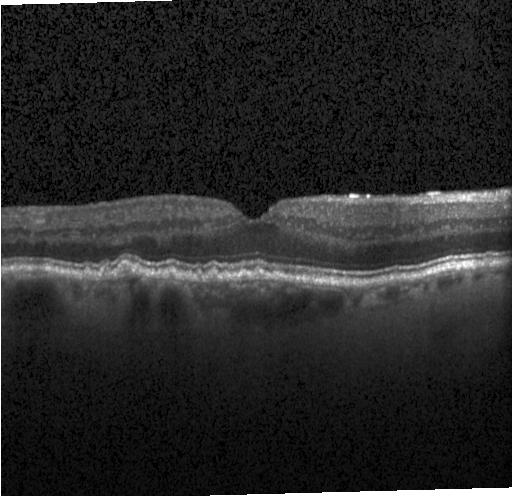
Retinal OCT B-scan · SD-OCT — Diagnosis: drusen.